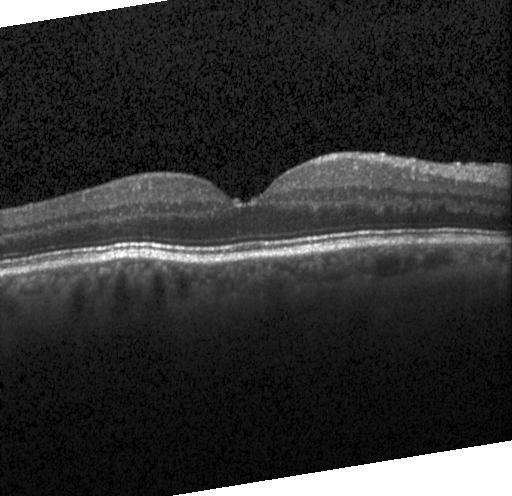
Diagnosis: no evidence of CNV, DME, or drusen.